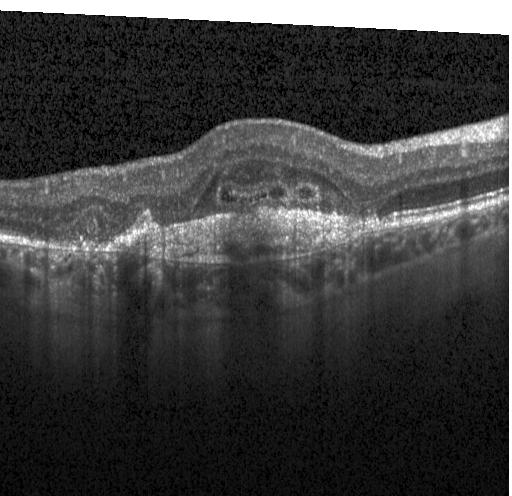

Optical coherence tomography B-scan. This B-scan demonstrates a choroidal neovascular membrane.